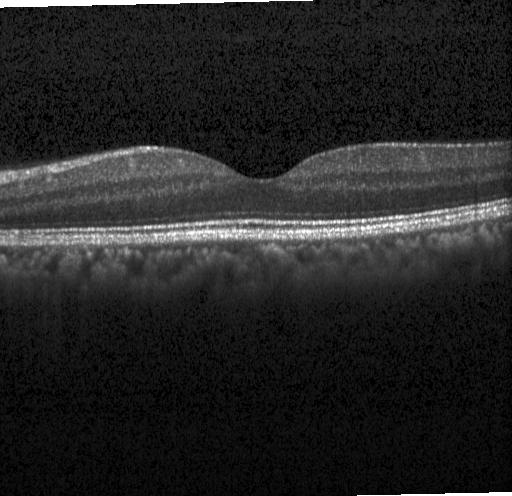 Retinal OCT cross-section showing neither choroidal neovascularization, diabetic macular edema, nor drusen.